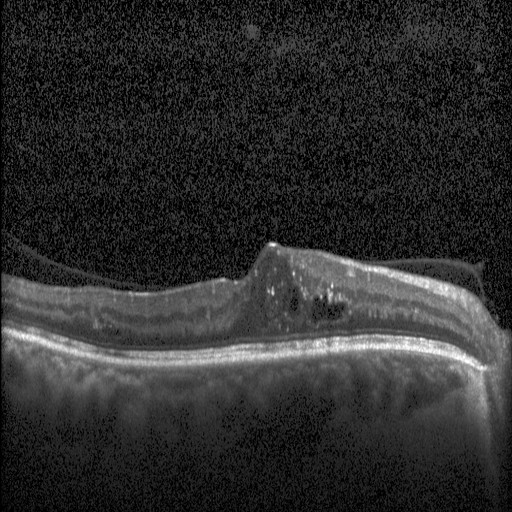 Impression: diabetic macular edema (DME).